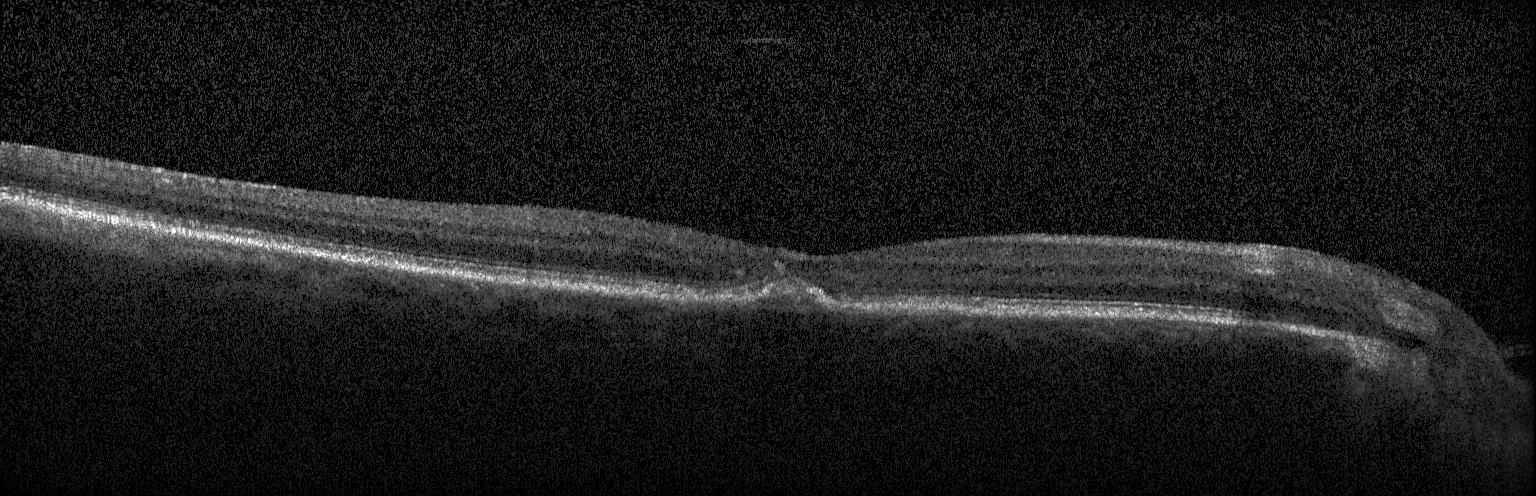
OCT B-scan showing a choroidal neovascular membrane.